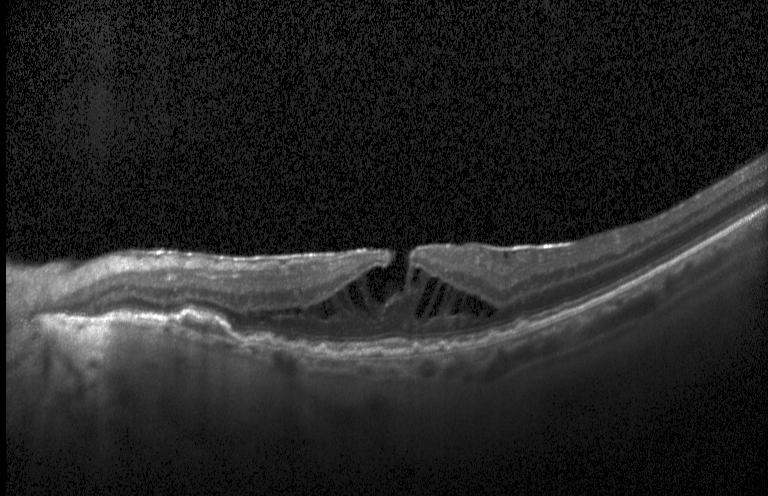 Retinal OCT cross-section
OCT finding: diabetic macular edema (DME).